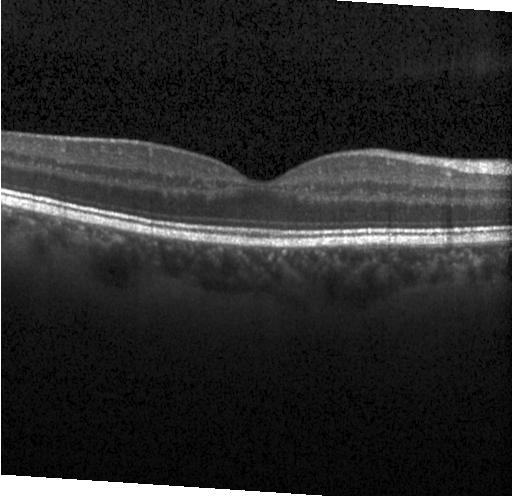 Retinal OCT cross-section · instrument: Heidelberg Spectralis · horizontal scan through the fovea.
This B-scan demonstrates no CNV, DME, or drusen.